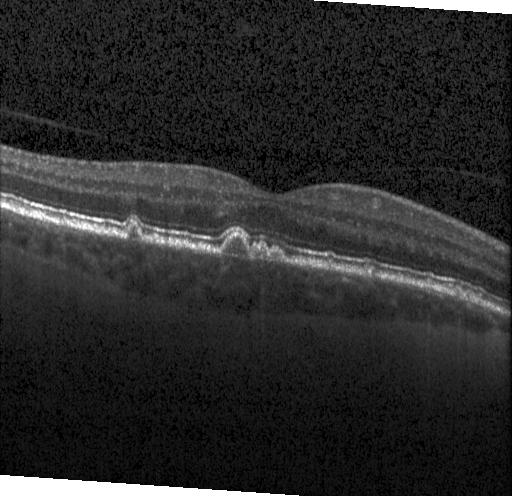
Spectral-domain OCT. Retinal OCT cross-section.
Diagnosis: drusen.